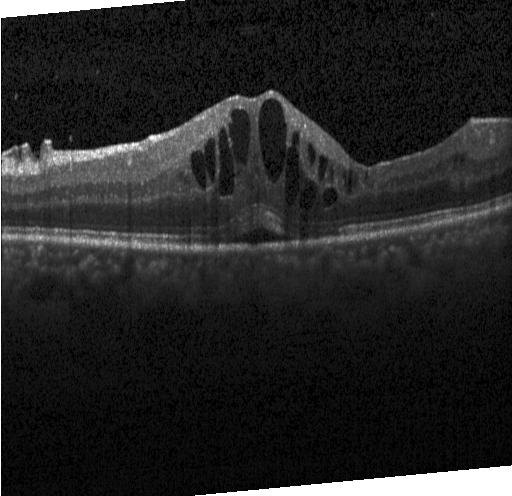
Through the macula, retinal OCT cross-section. Diagnosis: diabetic macular edema.